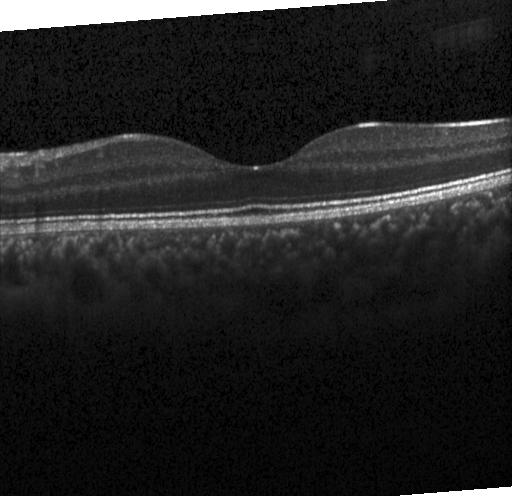
Macular OCT: no evidence of CNV, DME, or drusen.